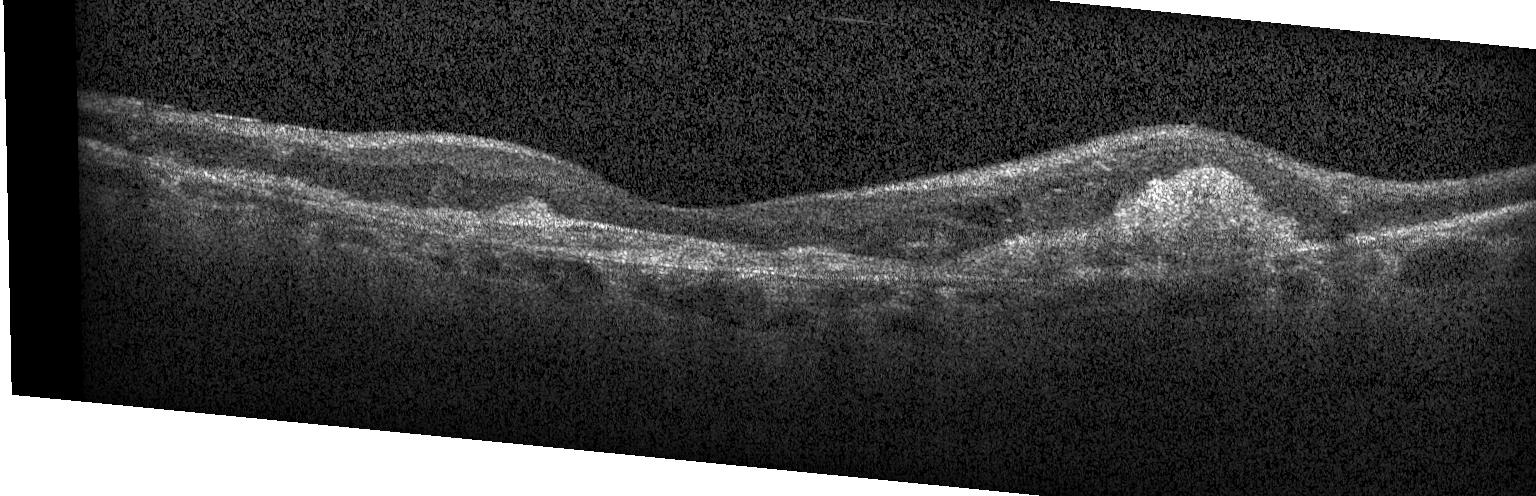 Optical coherence tomography scan · spectral-domain optical coherence tomography
The scan shows choroidal neovascularization.